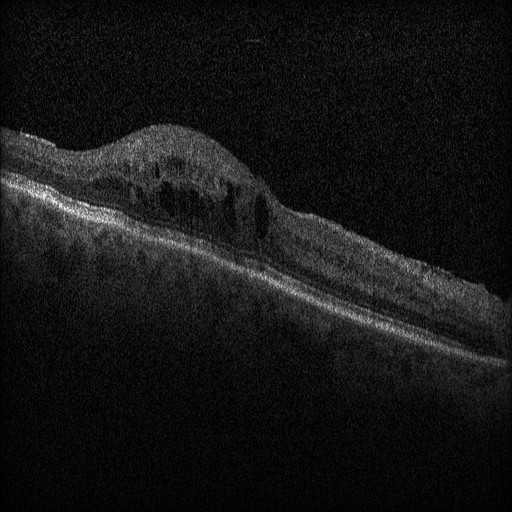 Retinal OCT cross-section. Finding: diabetic macular edema.